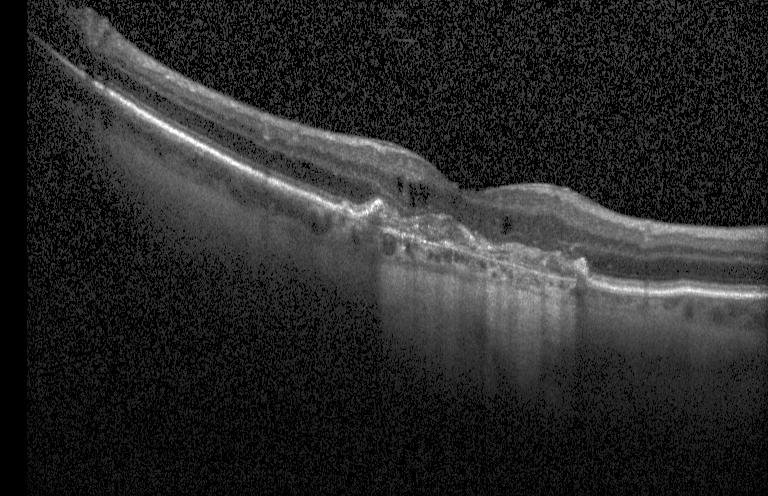
Retinal OCT B-scan — This B-scan demonstrates choroidal neovascularization.